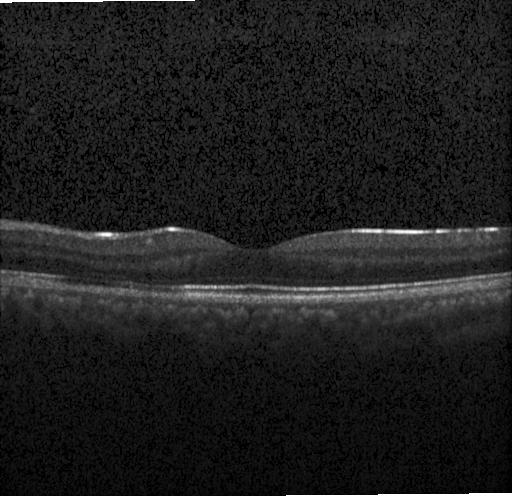 Diagnosis: no choroidal neovascularization, no diabetic macular edema, and no drusen.